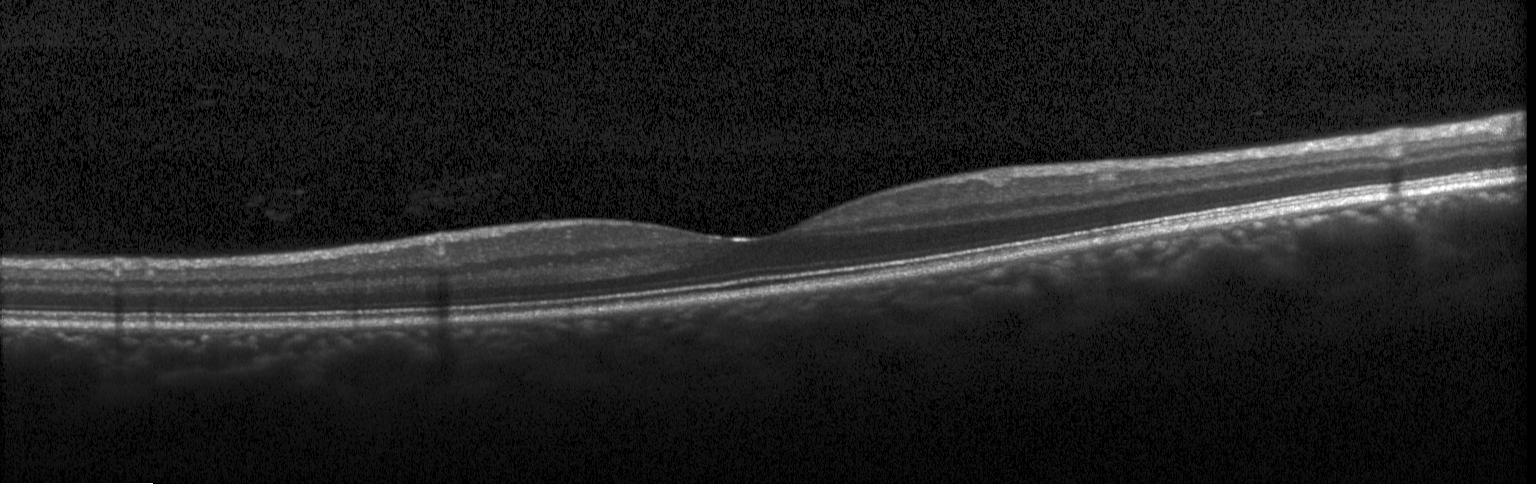
Impression: no evidence of choroidal neovascularization, diabetic macular edema, or drusen.